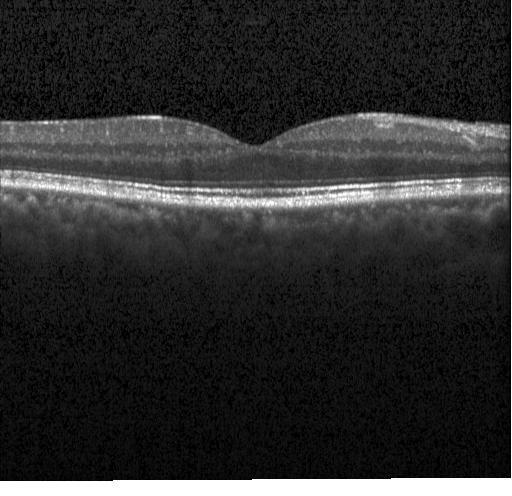
Impression: no CNV, no DME, and no drusen.